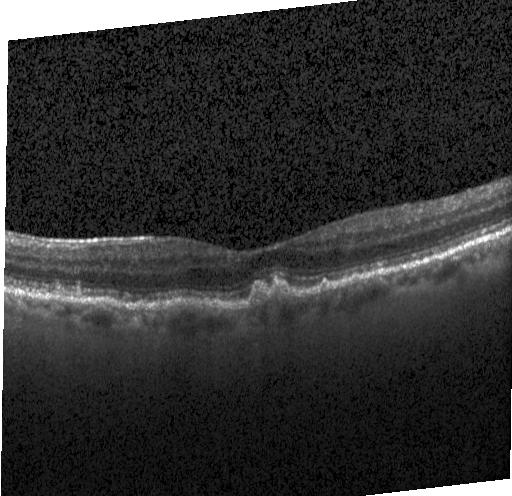

Heidelberg Spectralis OCT system; OCT line scan.
Multiple drusen.